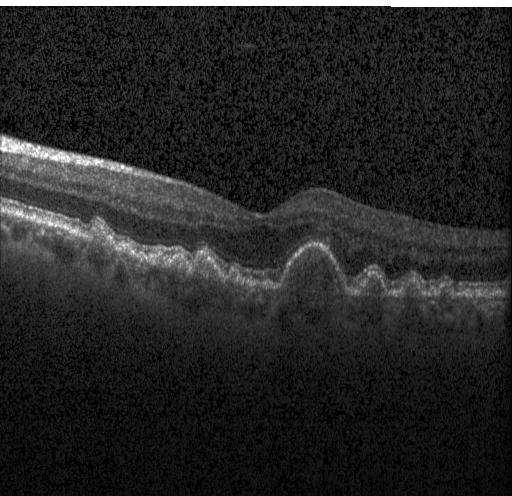

Retinal OCT B-scan.
Dx: sub-RPE drusenoid deposits.